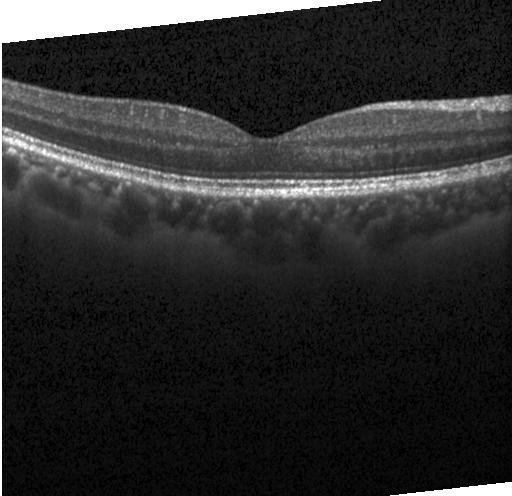
OCT finding: no choroidal neovascularization, diabetic macular edema, or drusen.